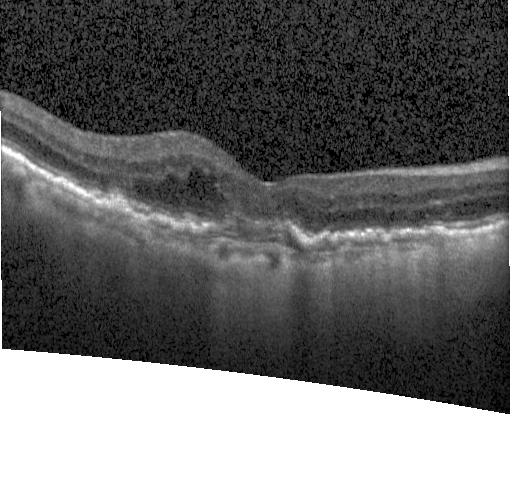

Impression: choroidal neovascularization (CNV).